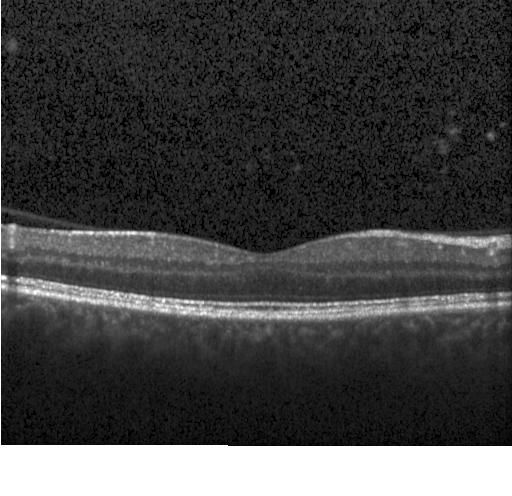

Impression: no evidence of choroidal neovascularization, diabetic macular edema, or drusen.